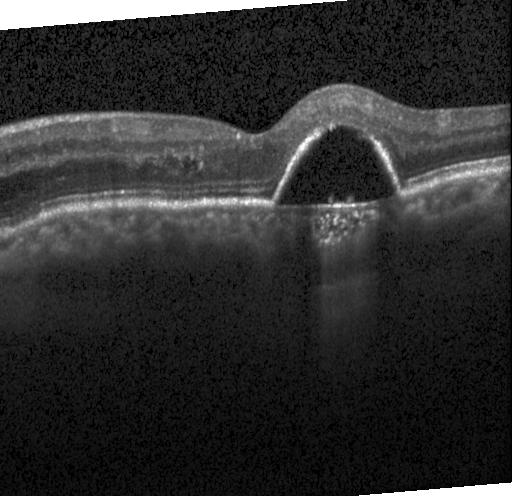

OCT line scan; instrument: Heidelberg Spectralis; macular scan. Finding: choroidal neovascularization (CNV).